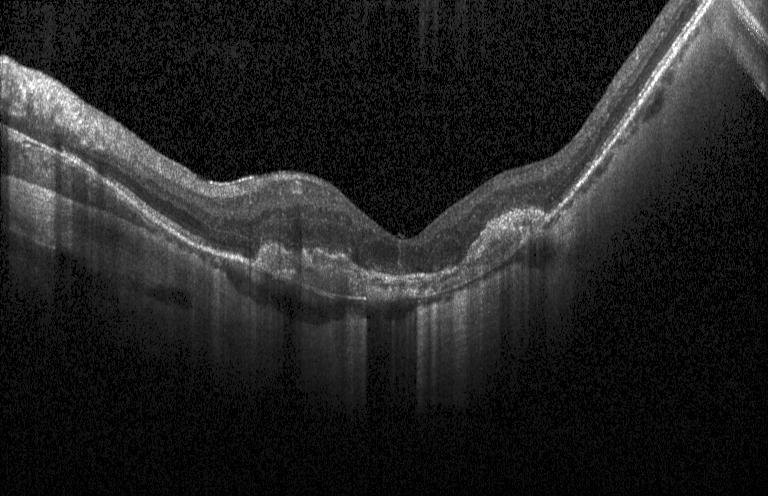
Optical coherence tomography B-scan, spectral-domain optical coherence tomography.
A choroidal neovascular membrane.